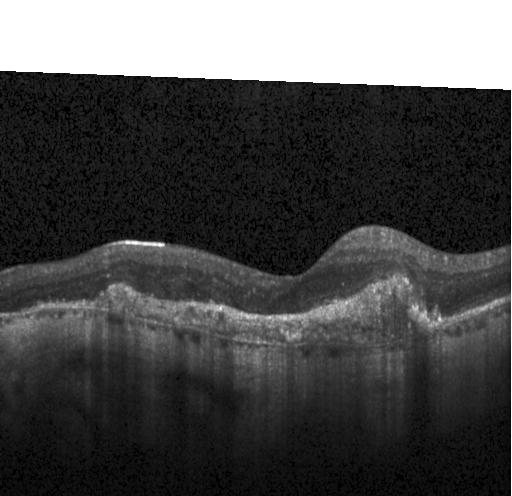 Acquired on a Heidelberg Spectralis; optical coherence tomography scan; spectral-domain OCT.
Impression: a choroidal neovascular membrane.